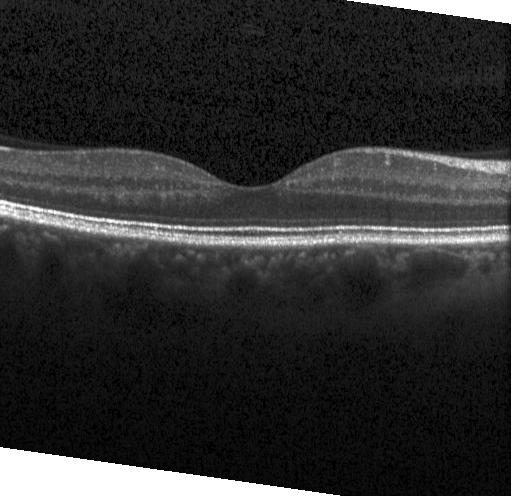

Instrument: Heidelberg Spectralis, fovea-centered, optical coherence tomography scan. Macular OCT: neither choroidal neovascularization, diabetic macular edema, nor drusen.